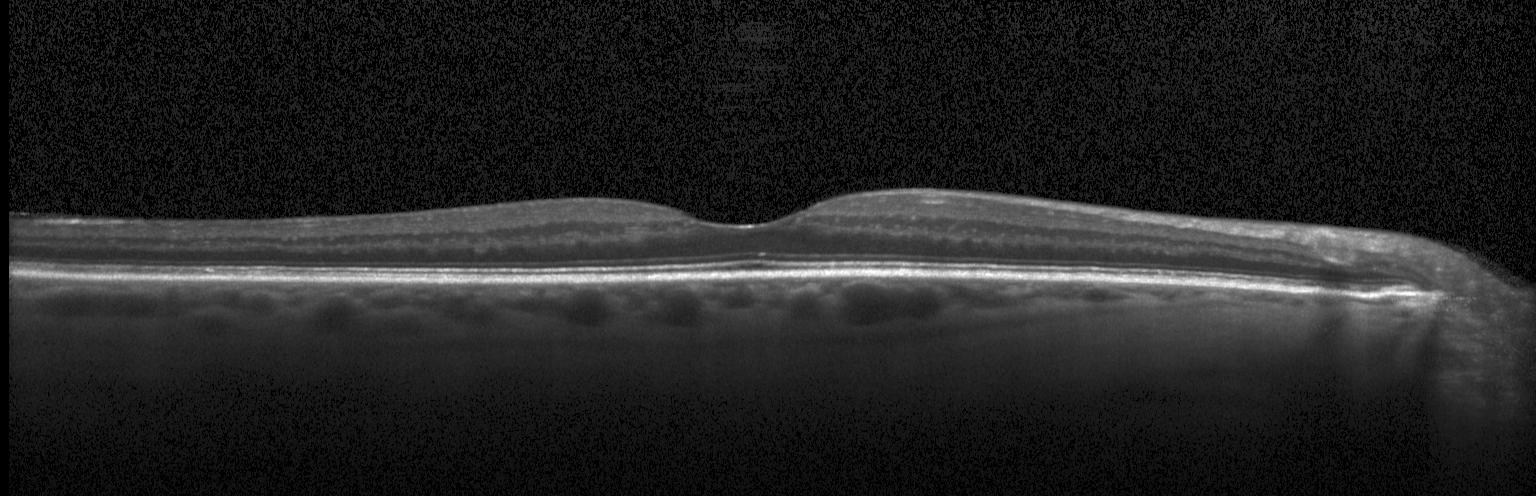 Optical coherence tomography B-scan · acquired on a Heidelberg Spectralis · SD-OCT. Assessment: neither CNV, DME, nor drusen.